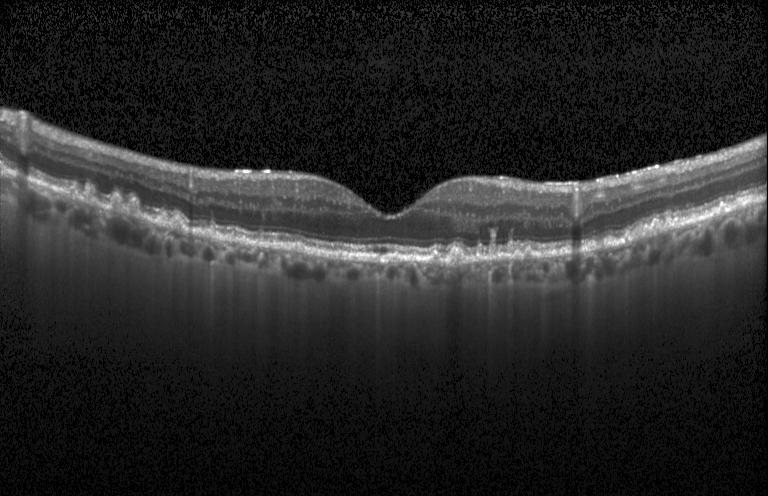

Macular scan · retinal OCT cross-section · Heidelberg Spectralis · spectral-domain OCT — The scan shows sub-RPE drusenoid deposits.